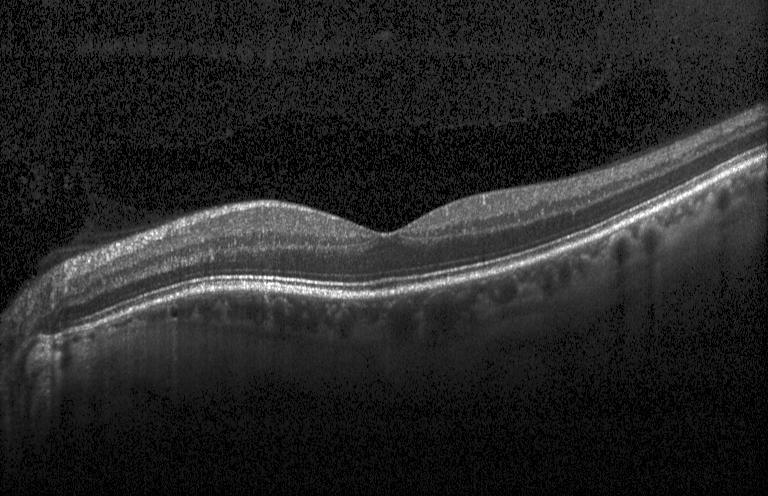

OCT line scan. Acquired on a Heidelberg Spectralis. Spectral-domain OCT. Horizontal scan through the fovea.
Assessment: no choroidal neovascularization, diabetic macular edema, or drusen.